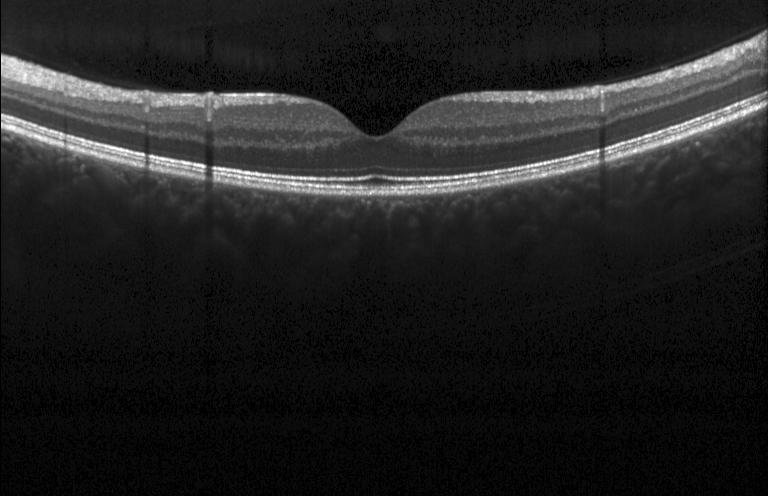

OCT B-scan. Finding: neither choroidal neovascularization, diabetic macular edema, nor drusen.